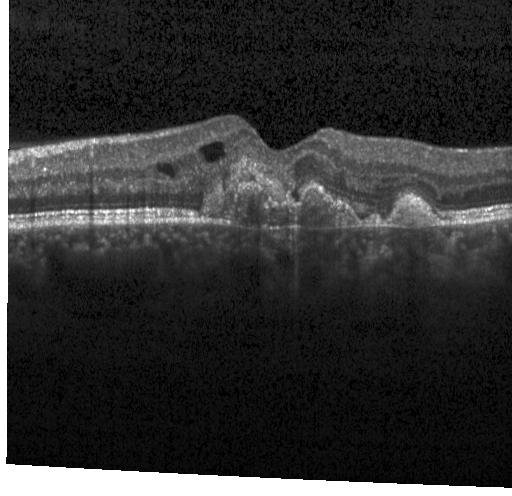
Optical coherence tomography scan. Assessment: a choroidal neovascular membrane.